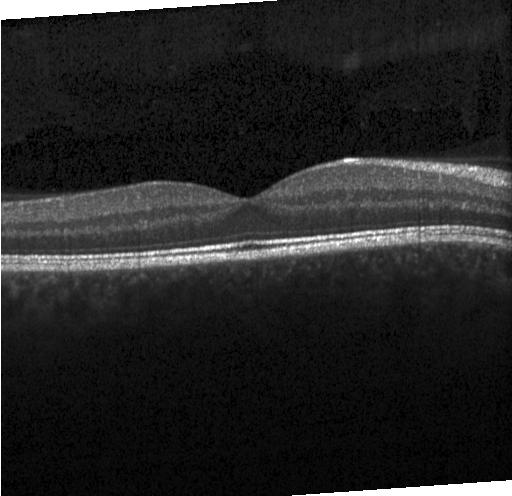
Dx: no choroidal neovascularization, no diabetic macular edema, and no drusen.